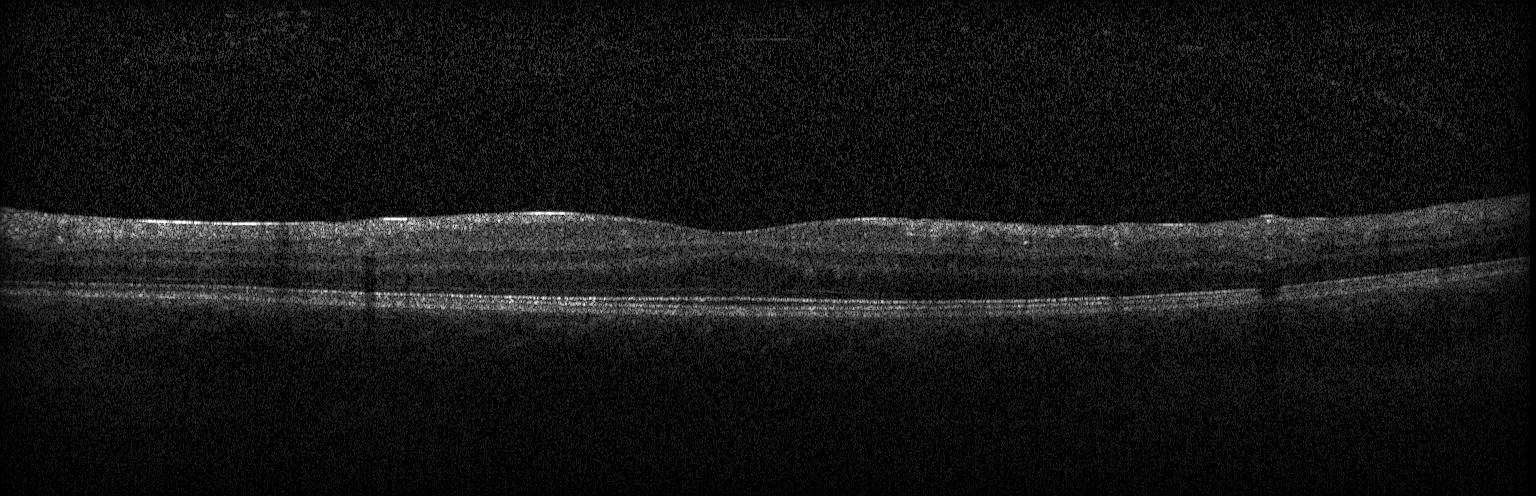 Acquired on a Heidelberg Spectralis, OCT line scan — Impression: neither choroidal neovascularization, diabetic macular edema, nor drusen.